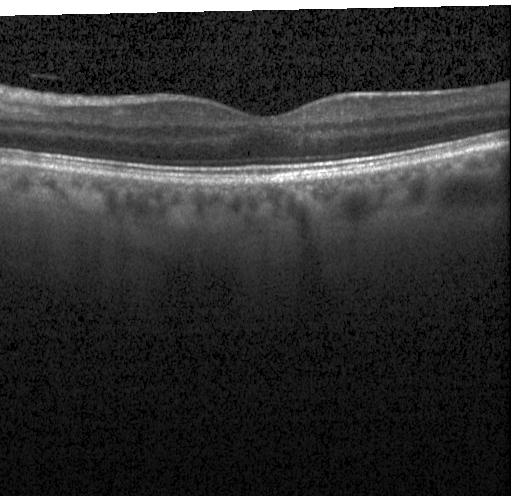

Finding: no evidence of choroidal neovascularization, diabetic macular edema, or drusen.